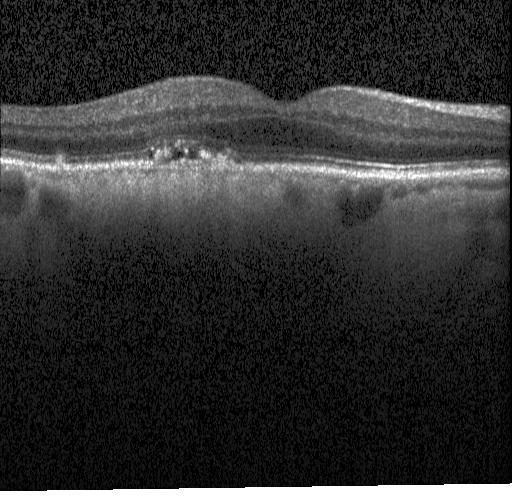
Finding: a choroidal neovascular membrane.